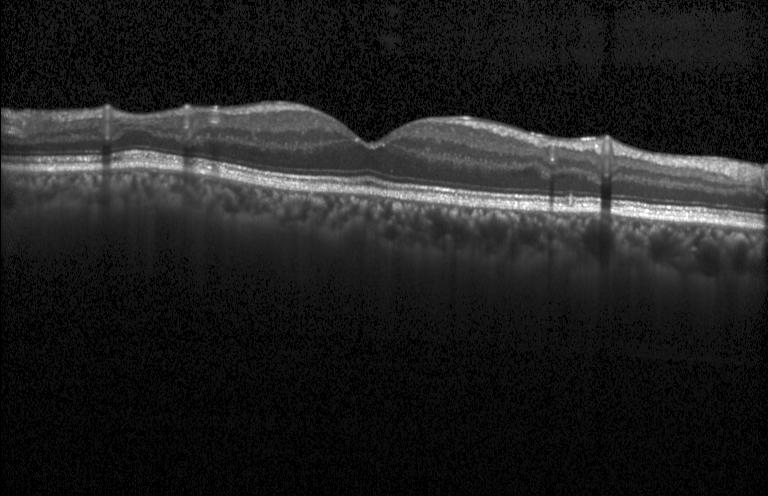 Spectral-domain OCT B-scan: neither choroidal neovascularization, diabetic macular edema, nor drusen.